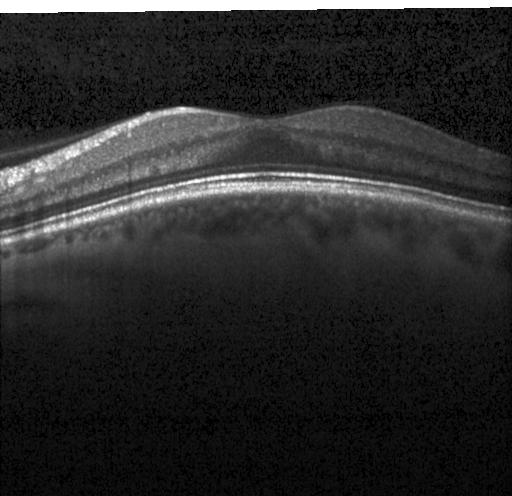 Neither CNV, DME, nor drusen.